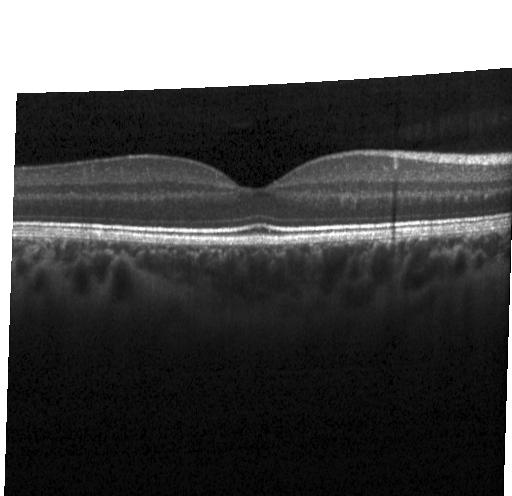 Acquired on a Heidelberg Spectralis · optical coherence tomography scan · horizontal scan through the fovea.
This B-scan demonstrates neither choroidal neovascularization, diabetic macular edema, nor drusen.